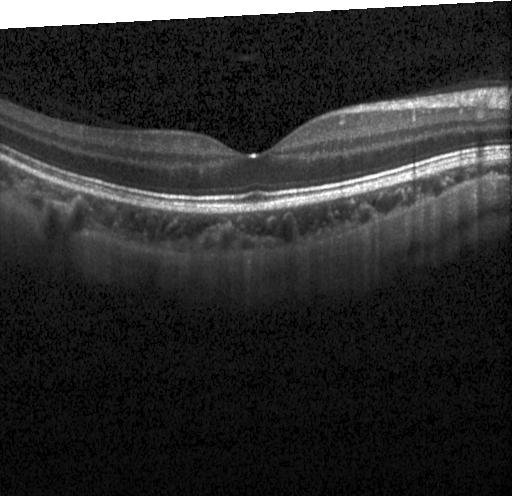

Spectral-domain optical coherence tomography; retinal OCT cross-section; fovea-centered.
Dx: no evidence of choroidal neovascularization, diabetic macular edema, or drusen.